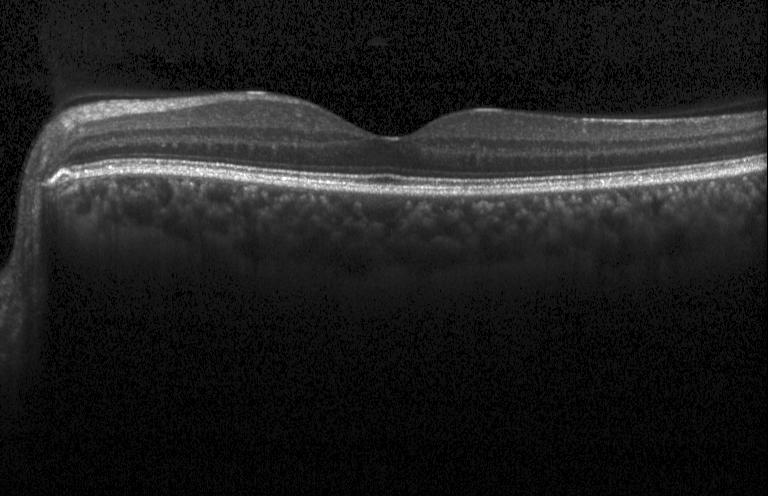

Optical coherence tomography scan
This B-scan demonstrates neither choroidal neovascularization, diabetic macular edema, nor drusen.